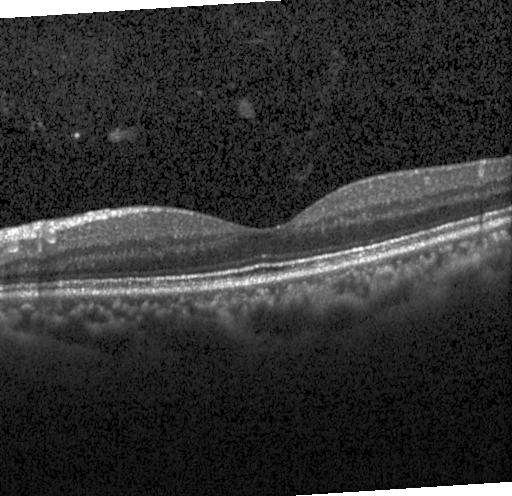
The scan shows neither choroidal neovascularization, diabetic macular edema, nor drusen.